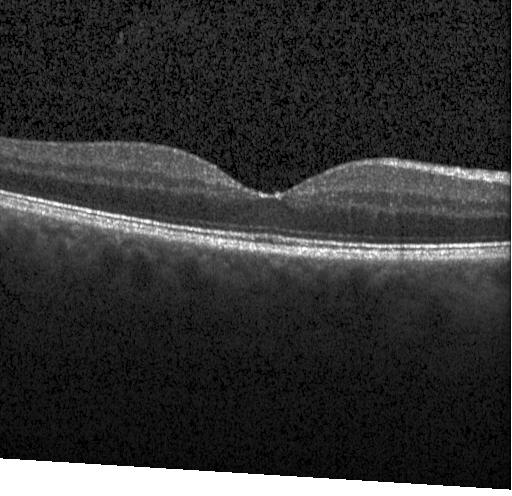
Optical coherence tomography B-scan. Fovea-centered.
Macular OCT: no evidence of CNV, DME, or drusen.